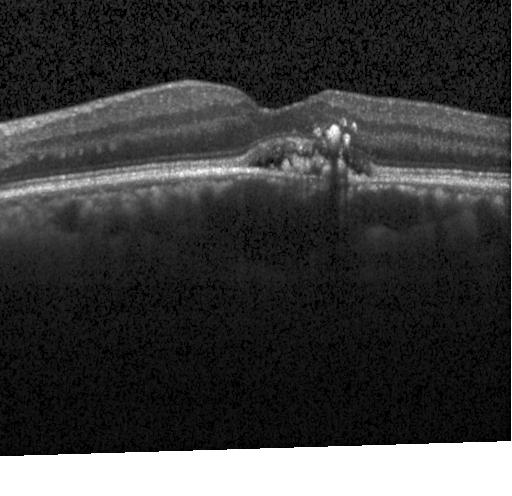
Optical coherence tomography B-scan, spectral-domain OCT. Assessment: a choroidal neovascular membrane.